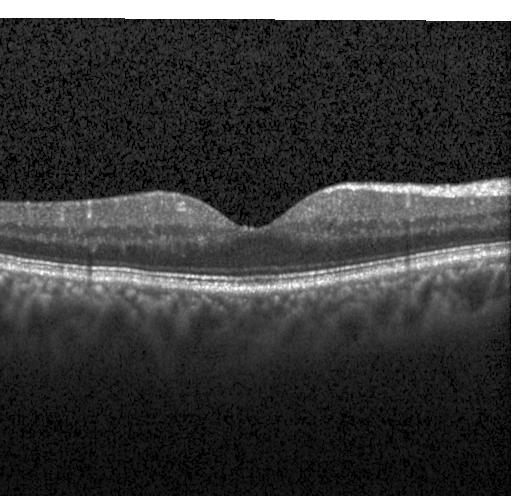
Fovea-centered · instrument: Heidelberg Spectralis · retinal OCT cross-section · SD-OCT. This B-scan demonstrates no evidence of CNV, DME, or drusen.